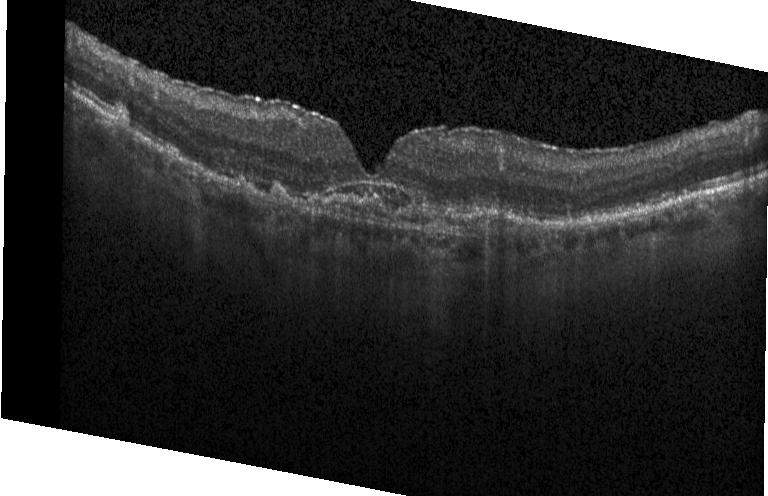

Centered on the fovea, SD-OCT, retinal OCT B-scan — Impression: choroidal neovascularization (CNV).